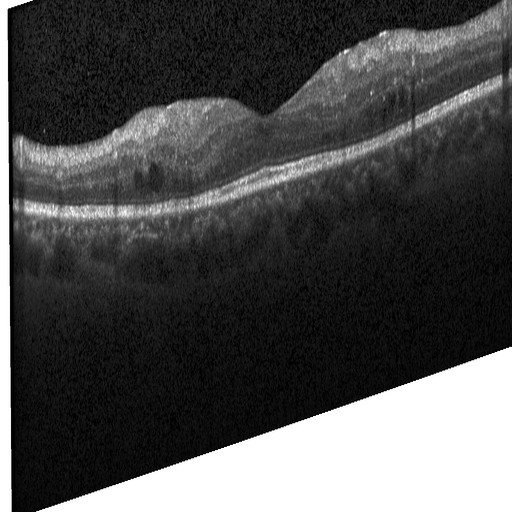

SD-OCT. Centered on the fovea. Optical coherence tomography B-scan. Heidelberg Spectralis.
Finding: diabetic macular edema (DME).